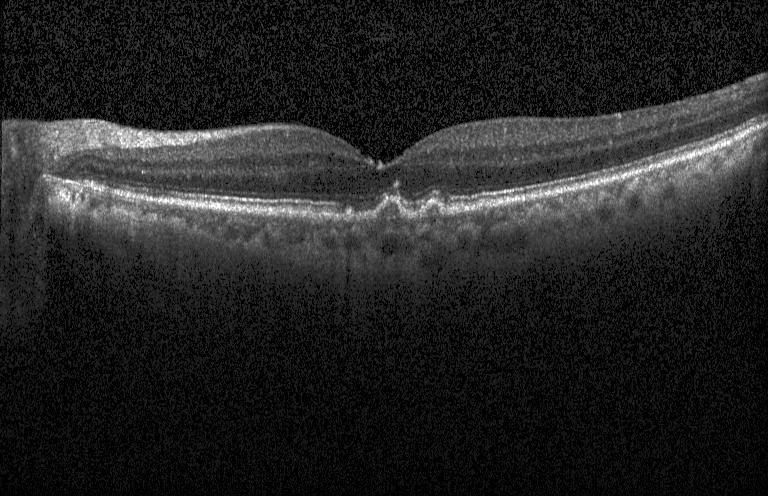

SD-OCT; through the macula; acquired on a Heidelberg Spectralis; OCT line scan. This B-scan demonstrates multiple drusen.